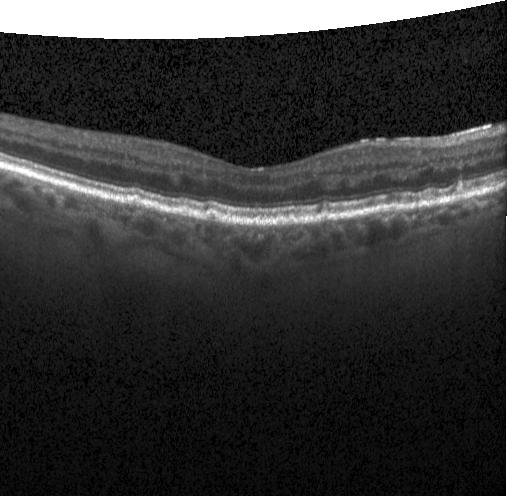 Diagnosis: sub-RPE drusenoid deposits.